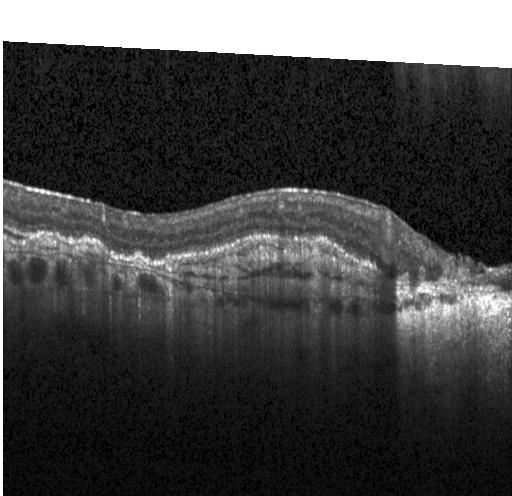

Optical coherence tomography B-scan. A choroidal neovascular membrane.